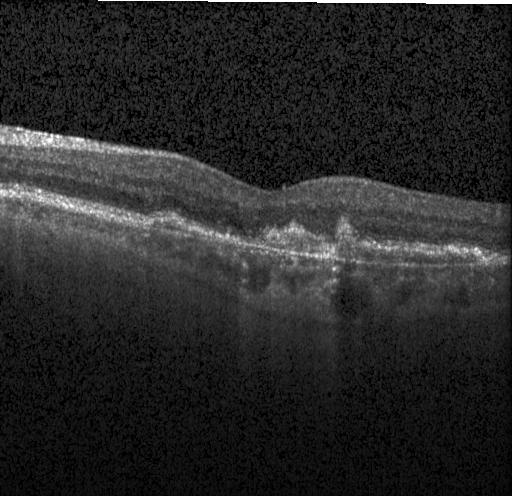

OCT line scan
Finding: a choroidal neovascular membrane.